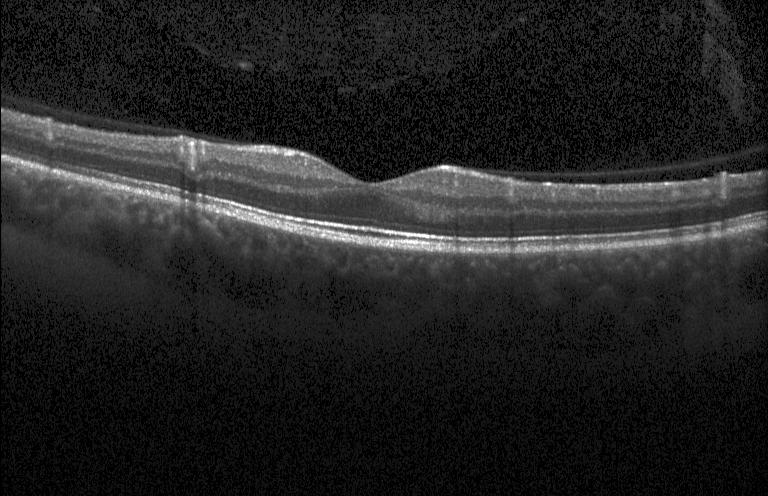

Diagnosis: no choroidal neovascularization, no diabetic macular edema, and no drusen.